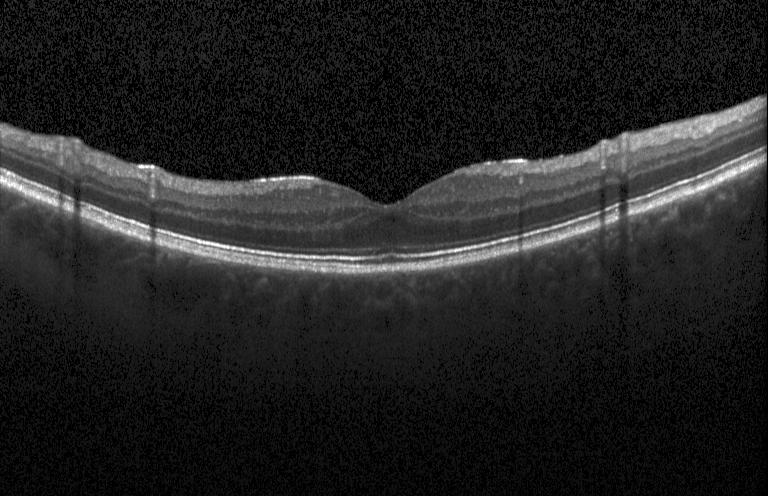 OCT B-scan. Fovea-centered. Heidelberg Spectralis OCT system — Assessment: no choroidal neovascularization, diabetic macular edema, or drusen.